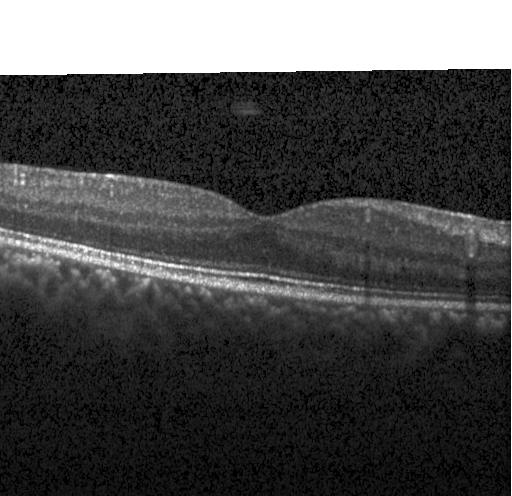
The scan shows neither choroidal neovascularization, diabetic macular edema, nor drusen.